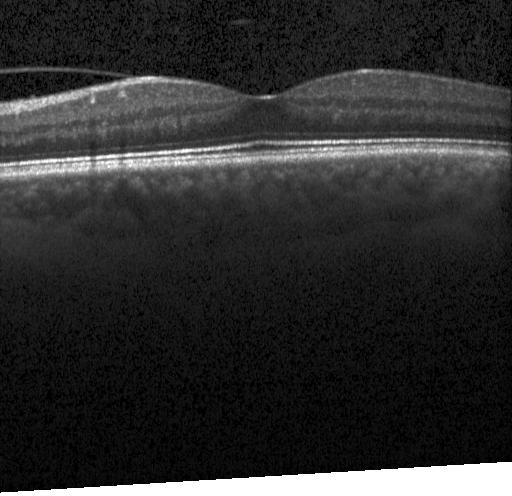

Diagnosis: no choroidal neovascularization, no diabetic macular edema, and no drusen.